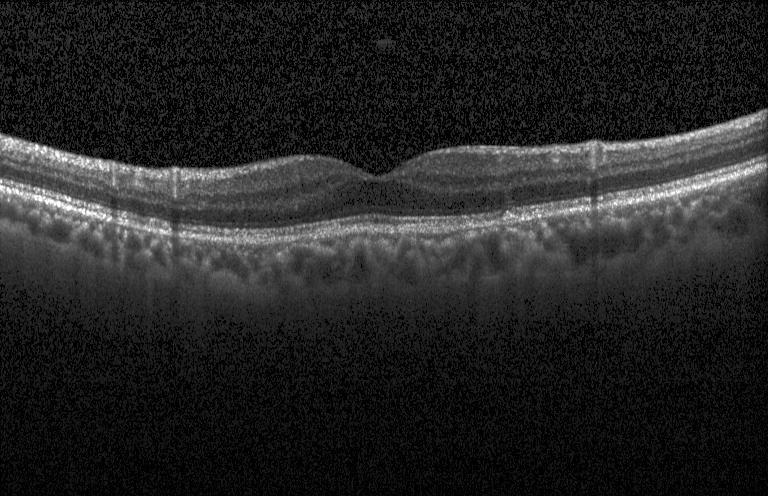

Optical coherence tomography B-scan; spectral-domain OCT
OCT finding: no CNV, no DME, and no drusen.